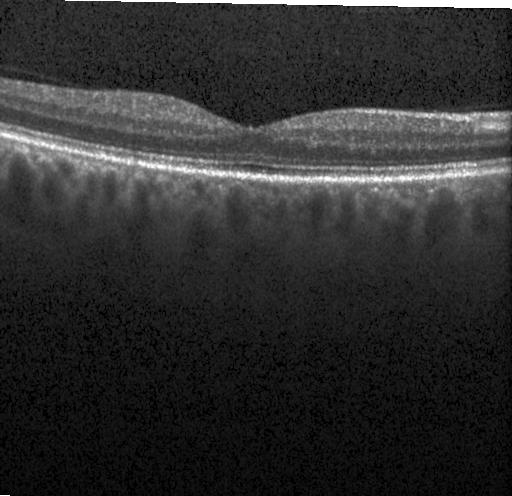

Heidelberg Spectralis · spectral-domain optical coherence tomography · macular scan · retinal OCT B-scan.
Impression: no choroidal neovascularization, no diabetic macular edema, and no drusen.